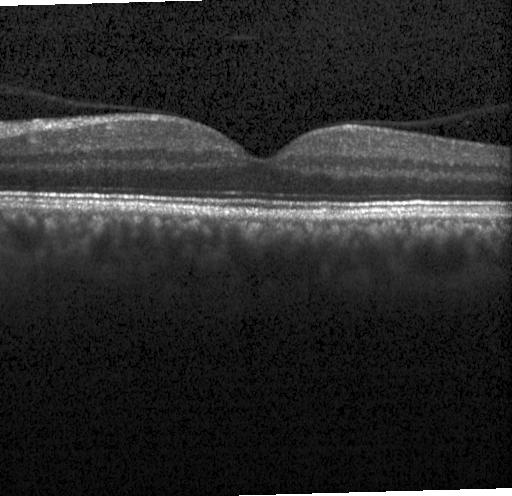

OCT B-scan showing no choroidal neovascularization, diabetic macular edema, or drusen.